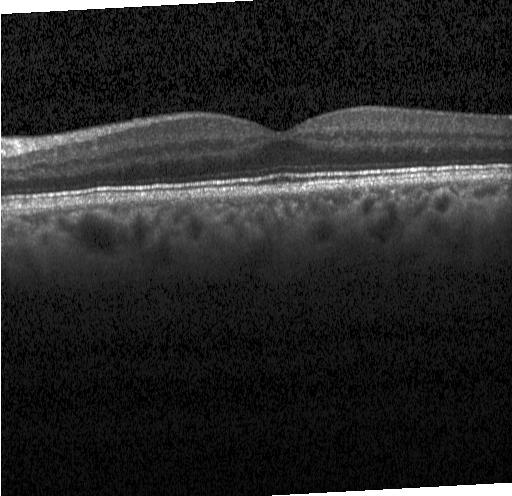
Impression: neither choroidal neovascularization, diabetic macular edema, nor drusen.